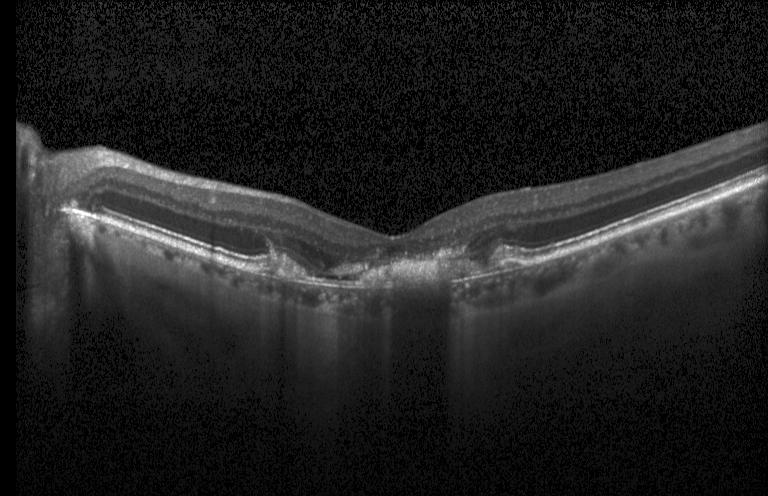
Spectral-domain OCT, retinal OCT cross-section, Heidelberg Spectralis, macular scan. The scan shows choroidal neovascularization.